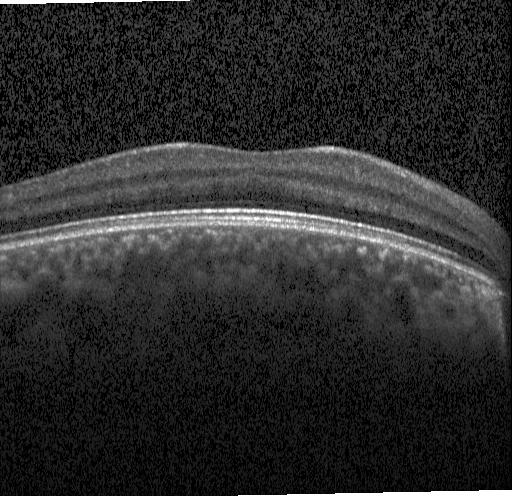 SD-OCT. Macular scan. Acquired on a Heidelberg Spectralis. OCT line scan.
Dx: no CNV, DME, or drusen.